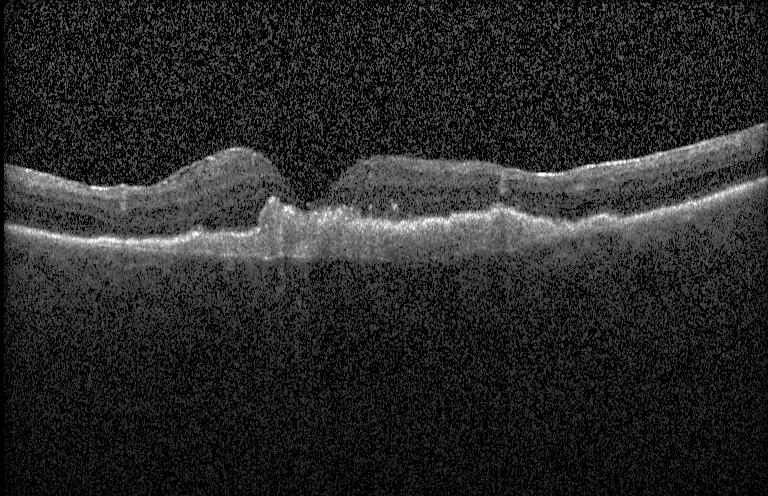
Acquired on a Heidelberg Spectralis · fovea-centered · retinal OCT cross-section.
The scan shows choroidal neovascularization (CNV).